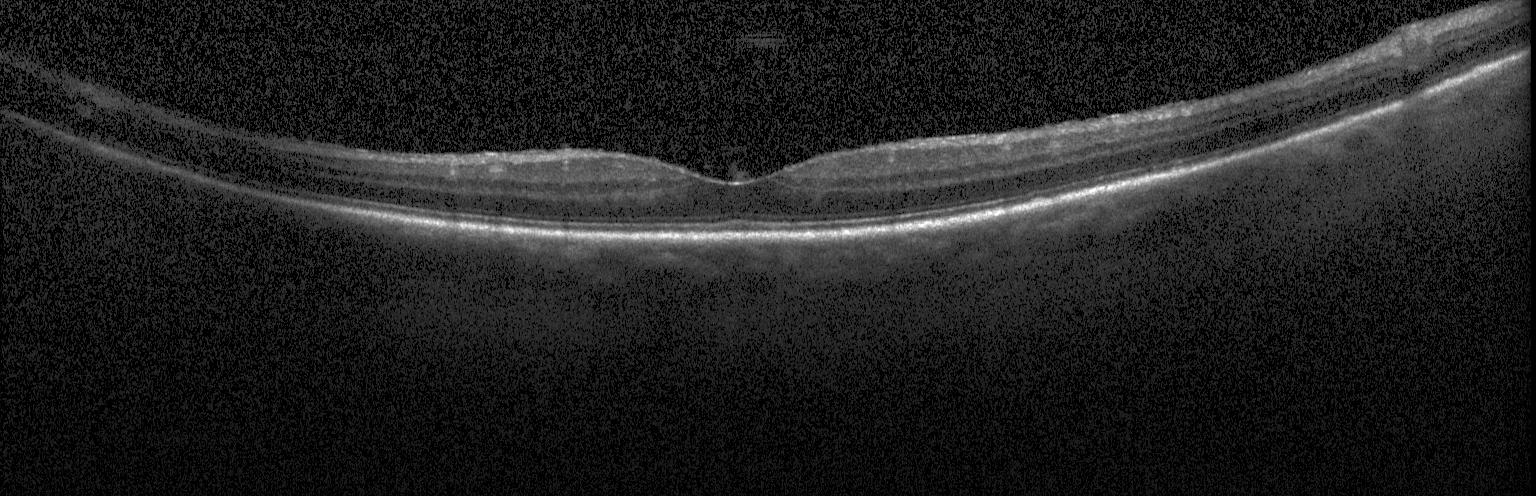
Impression: no CNV, DME, or drusen.